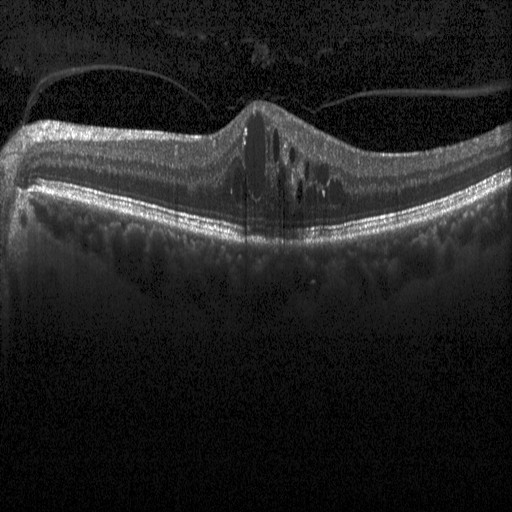
Finding: DME.